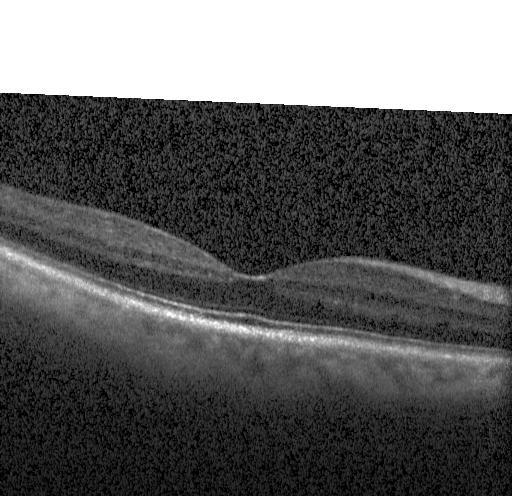 OCT scan showing neither choroidal neovascularization, diabetic macular edema, nor drusen.